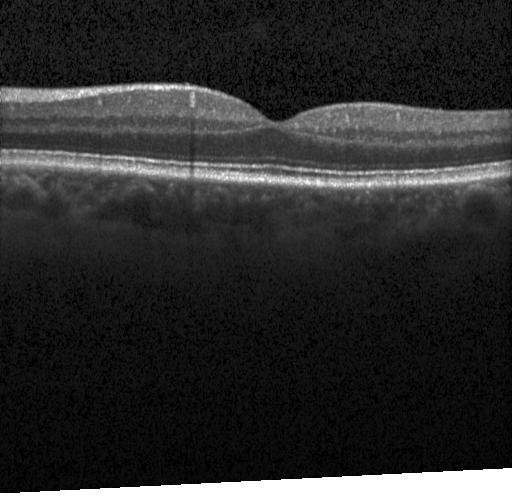
Heidelberg Spectralis OCT system, fovea-centered, OCT B-scan — This B-scan demonstrates neither CNV, DME, nor drusen.